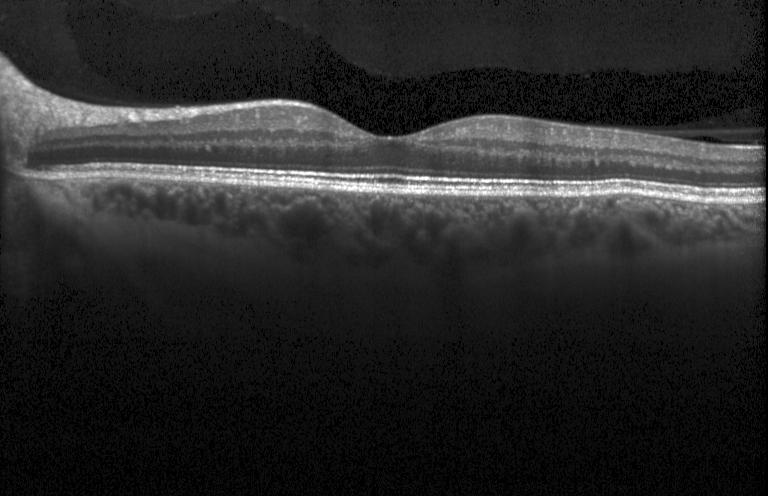
Optical coherence tomography scan · spectral-domain optical coherence tomography
Assessment: no evidence of choroidal neovascularization, diabetic macular edema, or drusen.